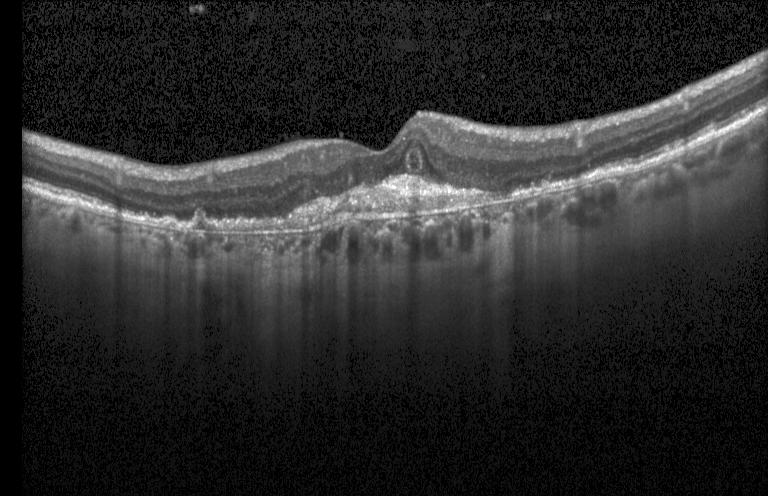
OCT B-scan. This B-scan demonstrates choroidal neovascularization (CNV).